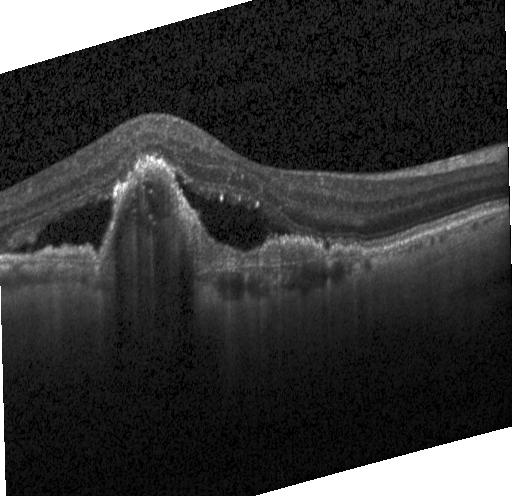
Impression: CNV.